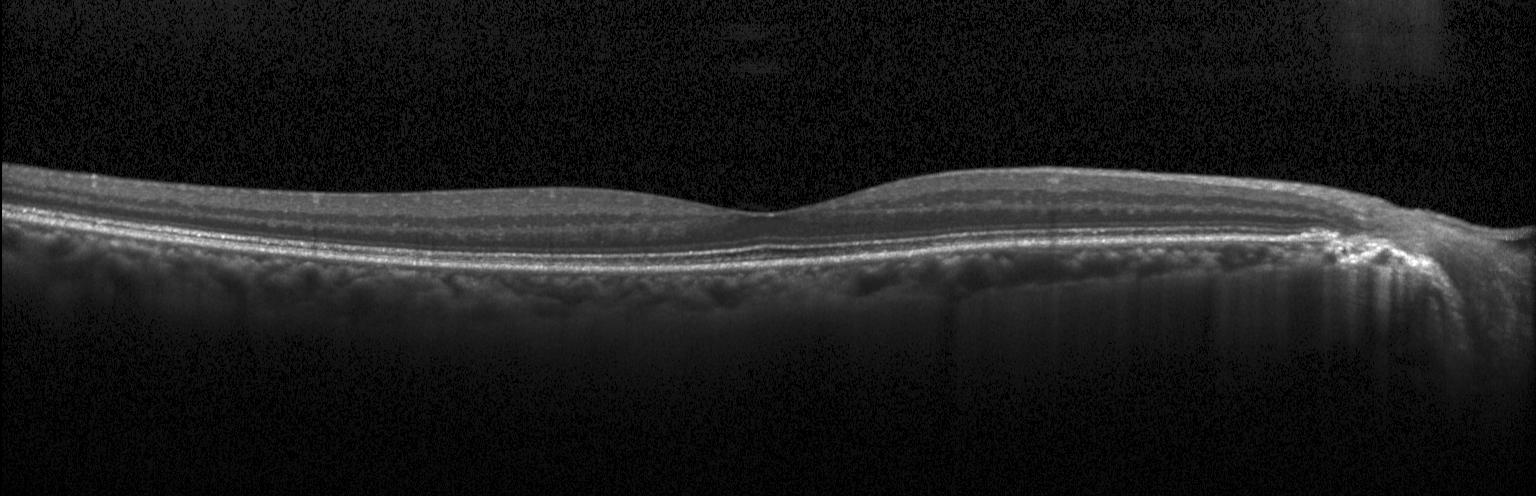 Retinal OCT B-scan
Diagnosis: no evidence of choroidal neovascularization, diabetic macular edema, or drusen.